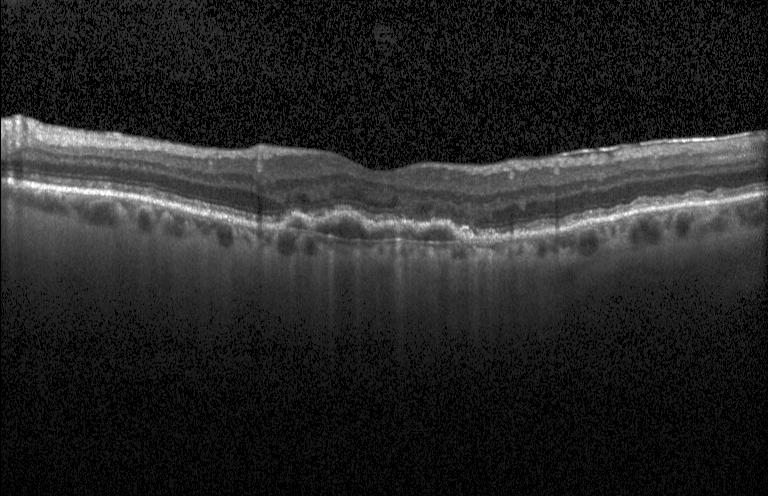 Acquired on a Heidelberg Spectralis. Centered on the fovea. Optical coherence tomography scan. Spectral-domain OCT
Finding: CNV.